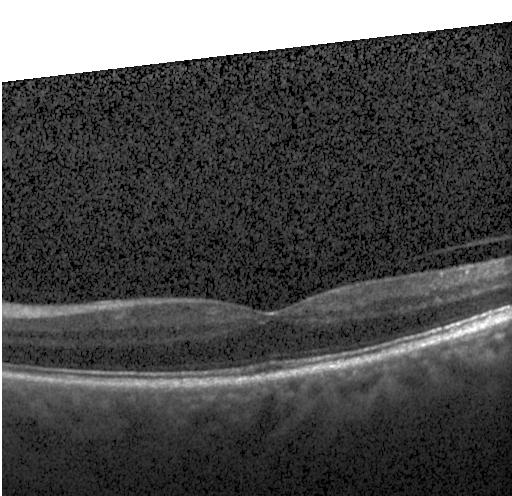 Dx: neither CNV, DME, nor drusen.